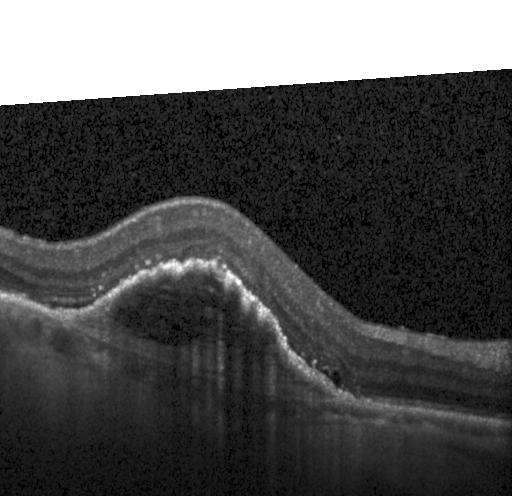 Finding: a choroidal neovascular membrane.